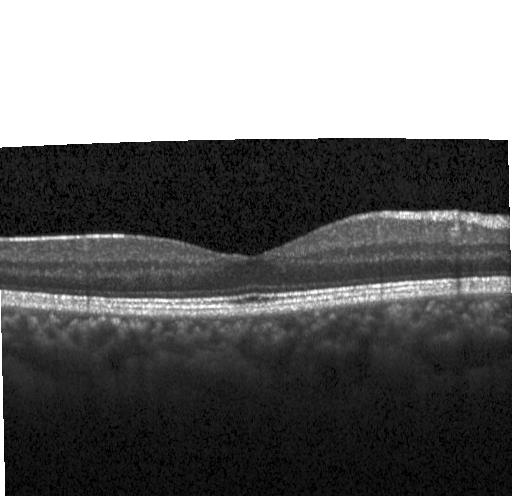 OCT line scan · spectral-domain OCT
Impression: no choroidal neovascularization, no diabetic macular edema, and no drusen.